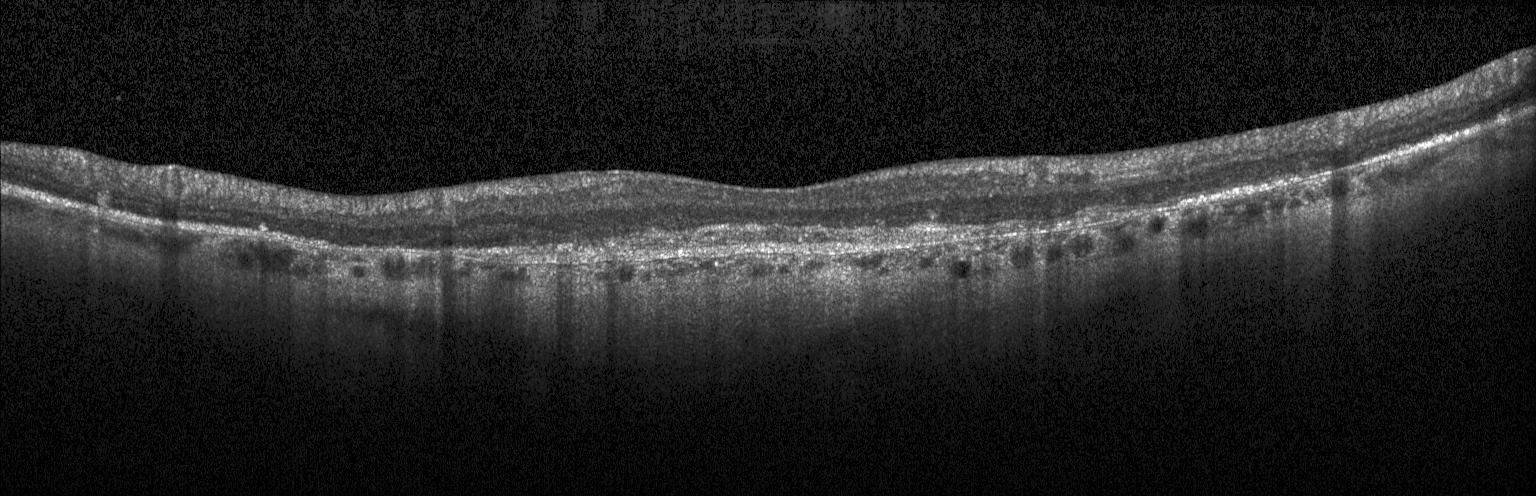

This B-scan demonstrates a choroidal neovascular membrane.